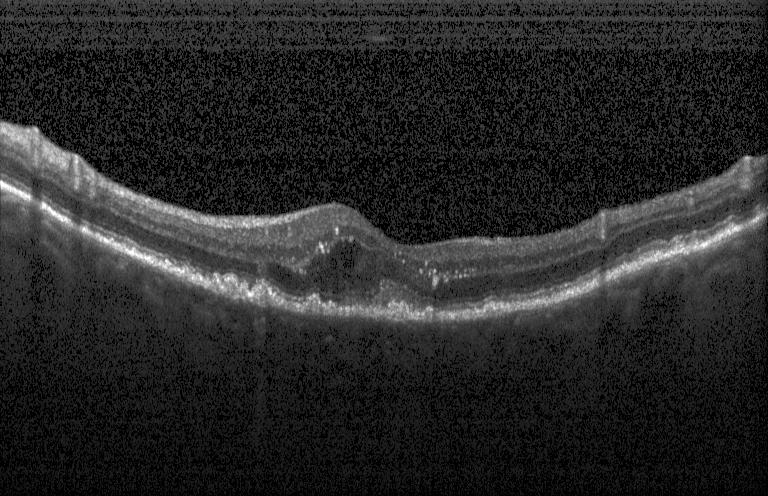 Spectral-domain OCT, Heidelberg Spectralis, macular scan, OCT line scan
This B-scan demonstrates CNV.